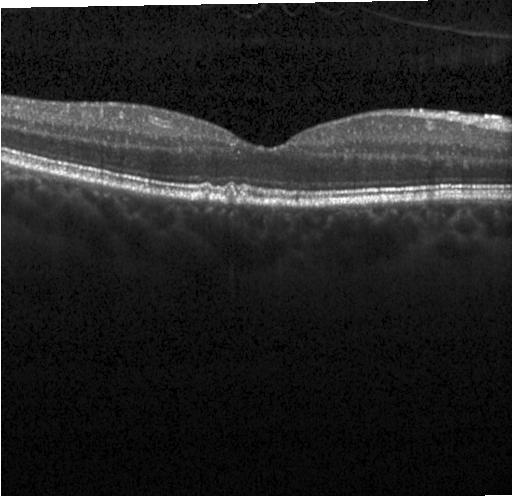 Optical coherence tomography B-scan; horizontal scan through the fovea; instrument: Heidelberg Spectralis. Assessment: drusen.